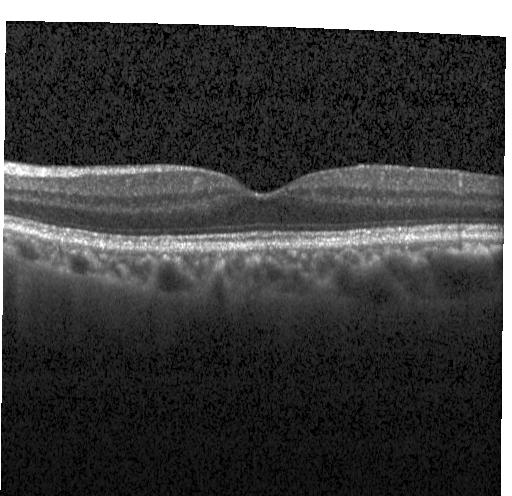
OCT B-scan, fovea-centered, Heidelberg Spectralis, spectral-domain OCT.
Impression: no evidence of CNV, DME, or drusen.